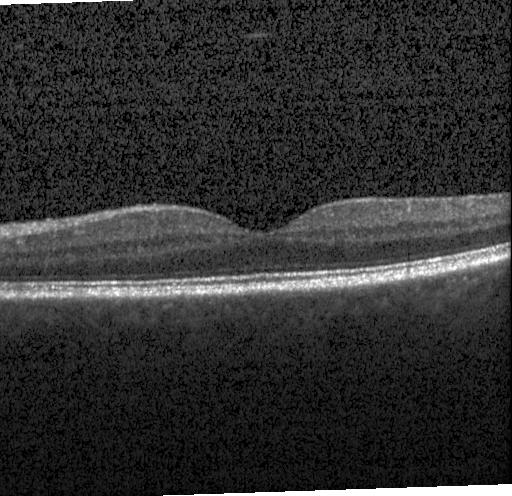 Retinal OCT cross-section showing no evidence of CNV, DME, or drusen.